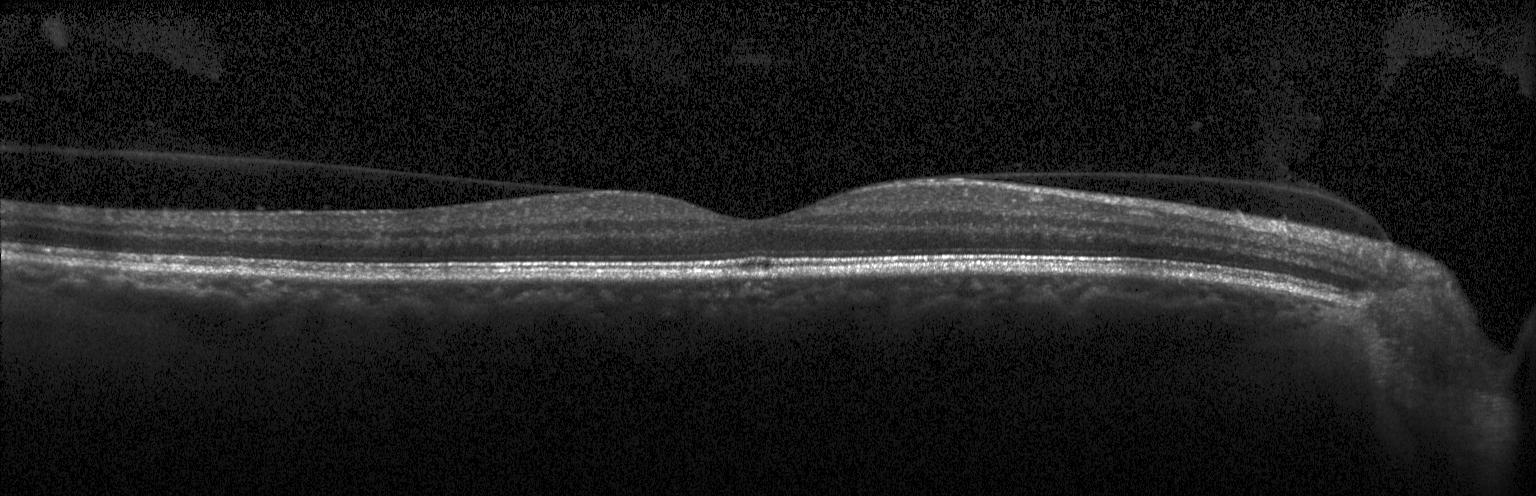 Heidelberg Spectralis, centered on the fovea, SD-OCT, optical coherence tomography B-scan. Finding: neither CNV, DME, nor drusen.